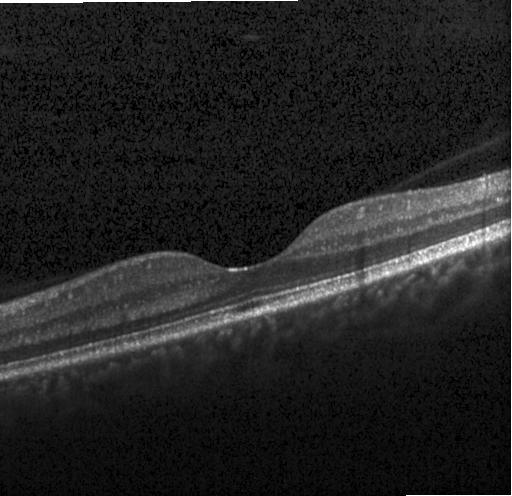
Dx: no evidence of CNV, DME, or drusen.